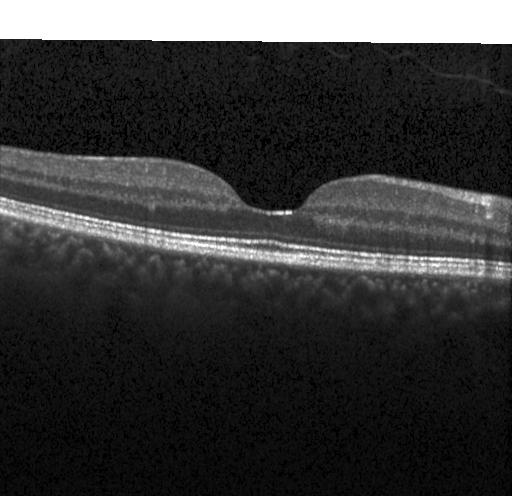 OCT B-scan, acquired on a Heidelberg Spectralis — Impression: no evidence of choroidal neovascularization, diabetic macular edema, or drusen.